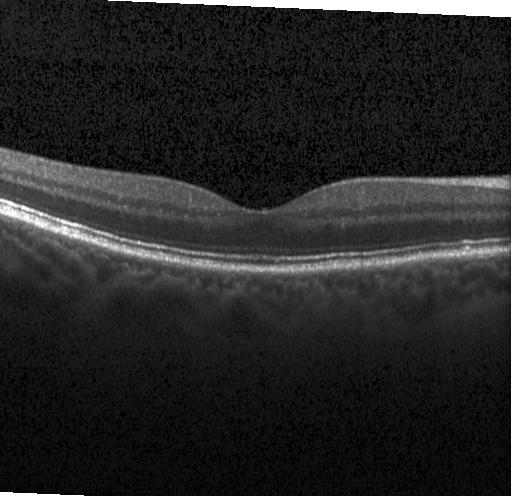

Macular OCT demonstrating no choroidal neovascularization, no diabetic macular edema, and no drusen.